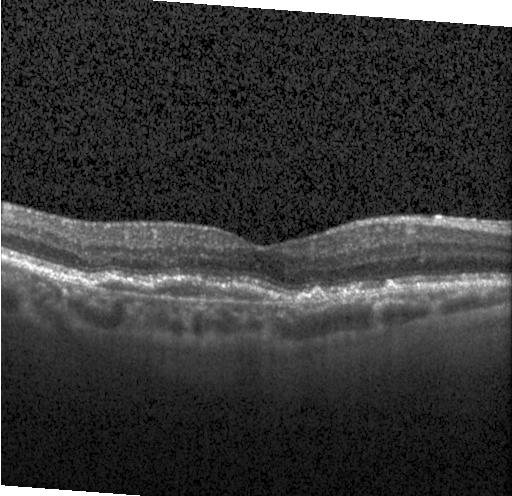
This B-scan demonstrates choroidal neovascularization (CNV).